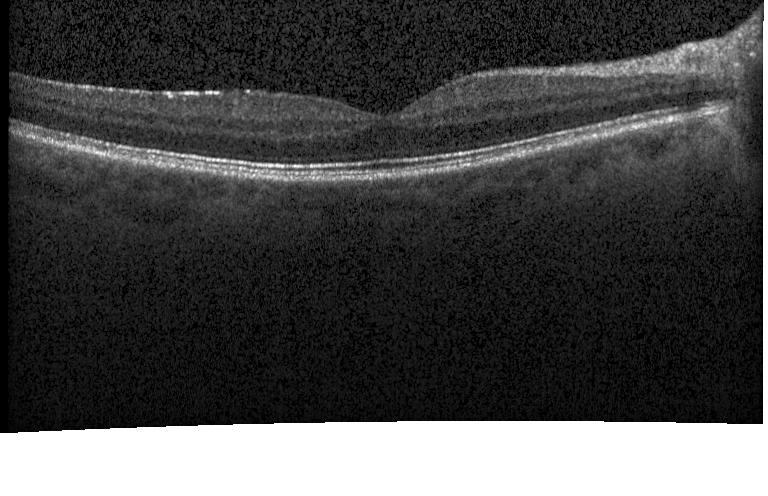

Centered on the fovea, spectral-domain optical coherence tomography, retinal OCT cross-section, acquired on a Heidelberg Spectralis. This B-scan demonstrates no CNV, no DME, and no drusen.